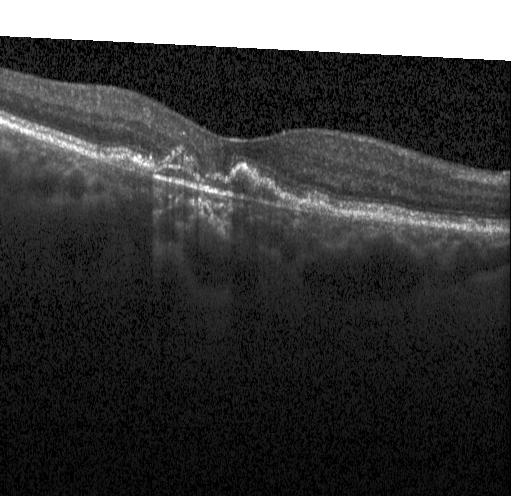
Dx: a choroidal neovascular membrane.